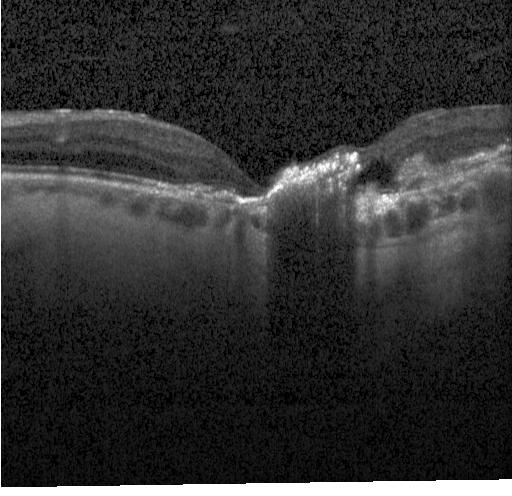
Heidelberg Spectralis · optical coherence tomography B-scan.
Assessment: a choroidal neovascular membrane.